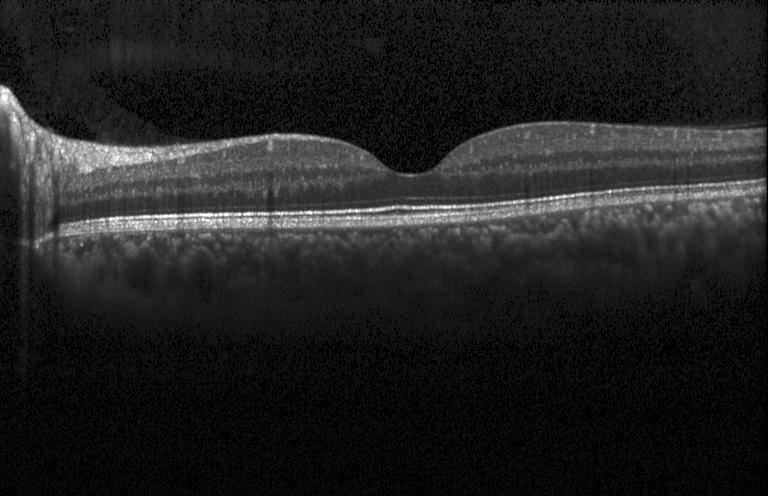

Spectral-domain optical coherence tomography, OCT B-scan, Heidelberg Spectralis OCT system. Diagnosis: neither choroidal neovascularization, diabetic macular edema, nor drusen.